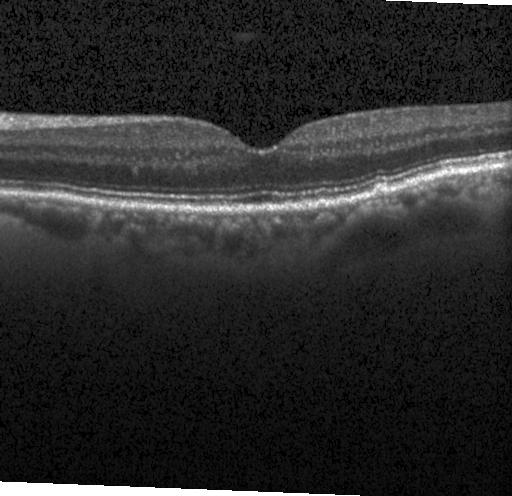 Acquired on a Heidelberg Spectralis; optical coherence tomography B-scan; spectral-domain OCT.
Sub-RPE drusenoid deposits.